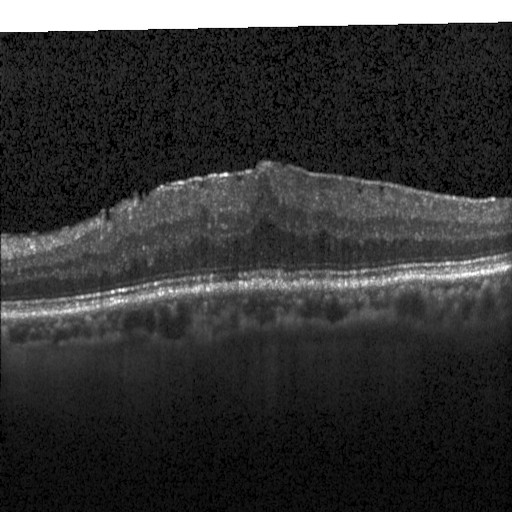 Retinal OCT cross-section, spectral-domain optical coherence tomography
The scan shows DME.